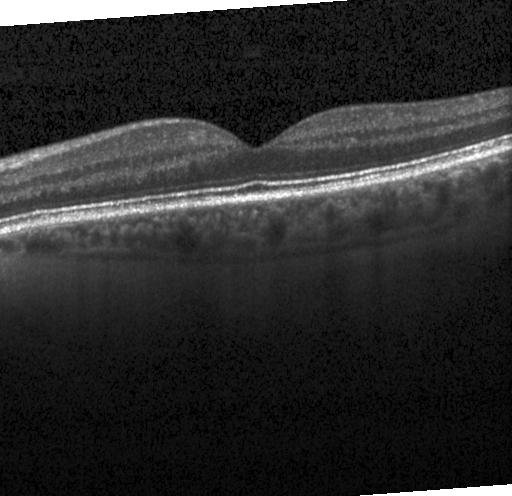

Finding: neither choroidal neovascularization, diabetic macular edema, nor drusen.